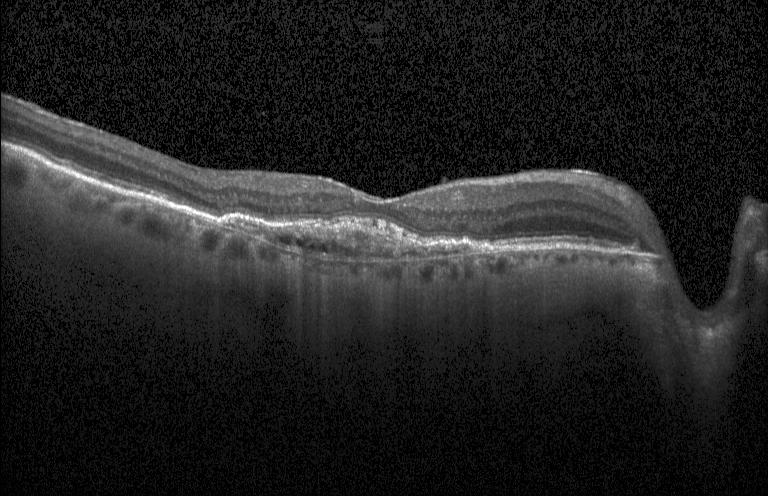

Acquired on a Heidelberg Spectralis · optical coherence tomography B-scan · SD-OCT. Impression: a choroidal neovascular membrane.